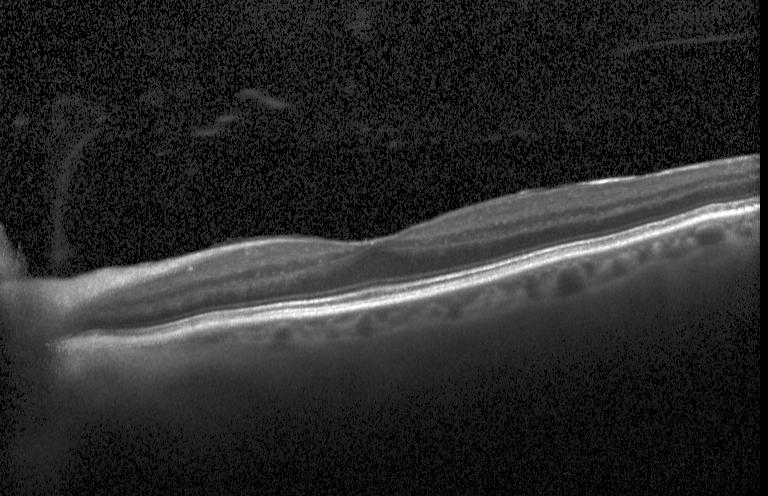 OCT finding: neither choroidal neovascularization, diabetic macular edema, nor drusen.